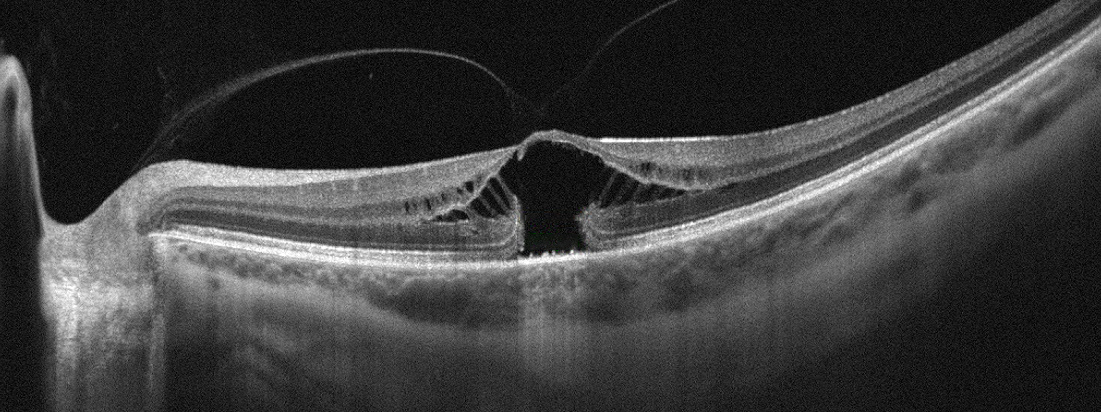

OCT B-scan — Macular OCT: vitreomacular interface disease.